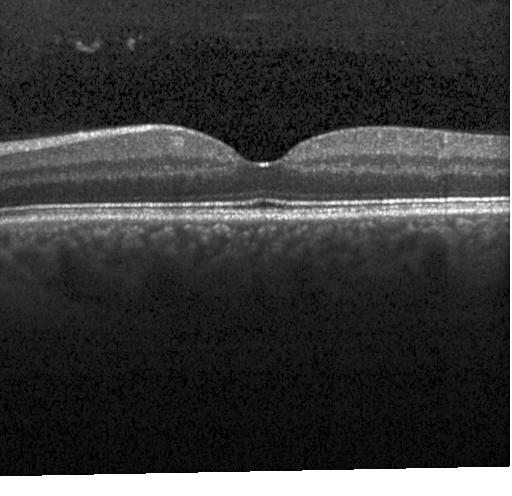
OCT line scan. Acquired on a Heidelberg Spectralis. Centered on the fovea. Spectral-domain OCT. Dx: no evidence of choroidal neovascularization, diabetic macular edema, or drusen.